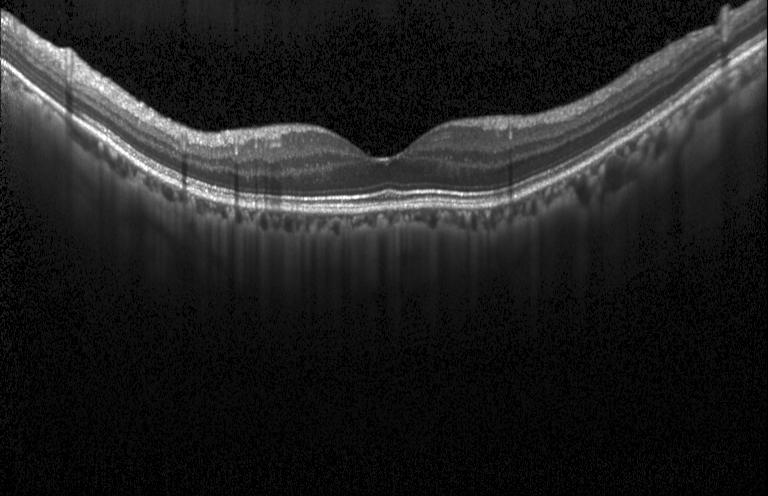

Optical coherence tomography scan · SD-OCT · Heidelberg Spectralis — Dx: no CNV, no DME, and no drusen.